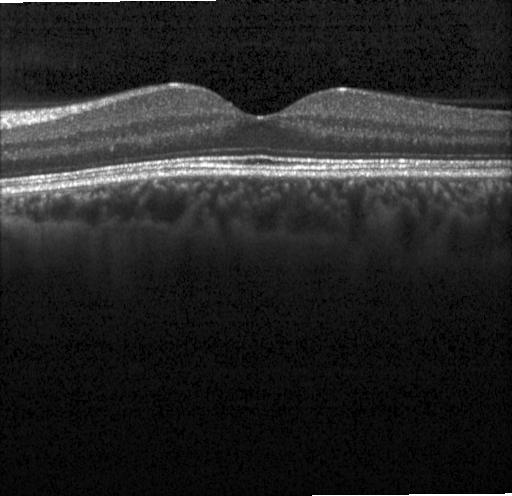

Heidelberg Spectralis OCT system; retinal OCT B-scan; through the macula. Diagnosis: no CNV, DME, or drusen.